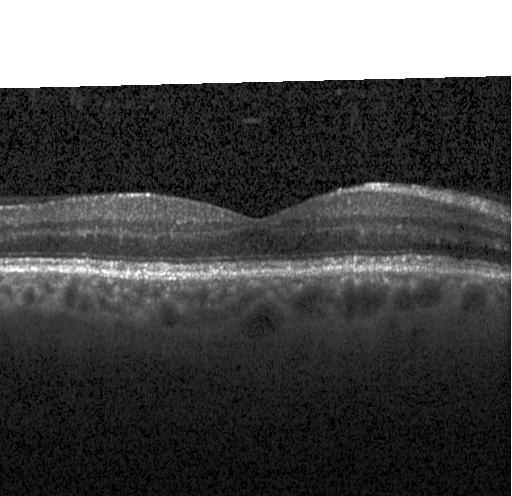
Spectral-domain optical coherence tomography. Fovea-centered. Optical coherence tomography scan. Impression: no evidence of choroidal neovascularization, diabetic macular edema, or drusen.